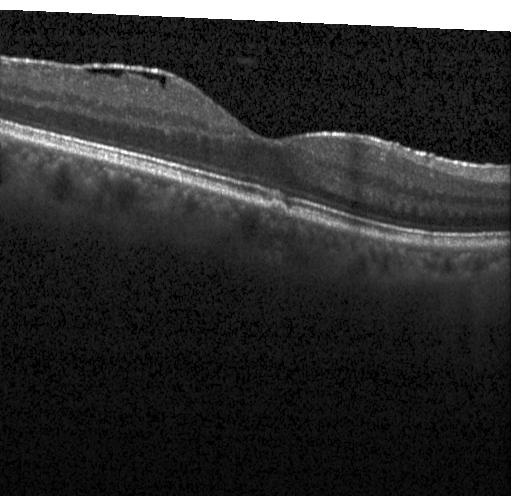
Spectral-domain optical coherence tomography · acquired on a Heidelberg Spectralis · retinal OCT cross-section · through the macula — The scan shows multiple drusen.